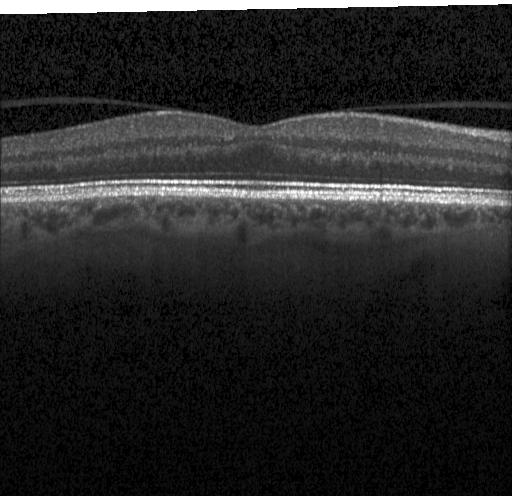

Acquired on a Heidelberg Spectralis · optical coherence tomography scan — Diagnosis: neither choroidal neovascularization, diabetic macular edema, nor drusen.